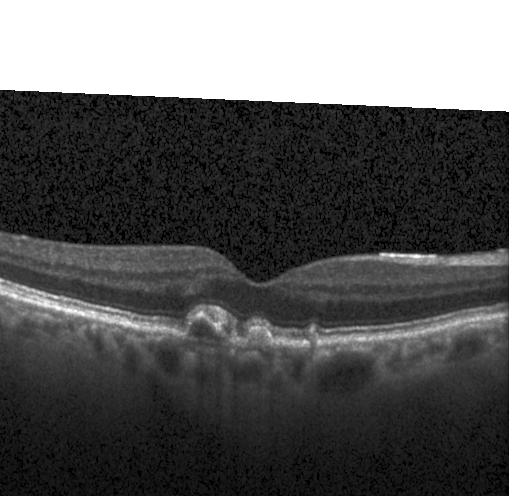 Macular OCT demonstrating choroidal neovascularization (CNV).